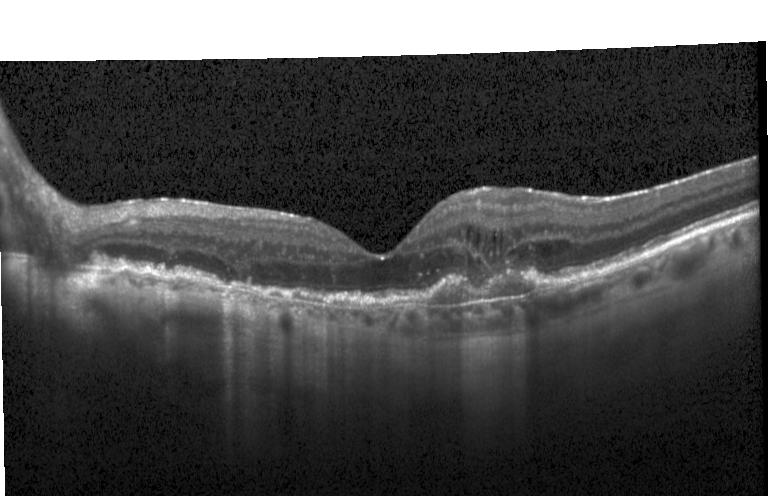 Impression: a choroidal neovascular membrane.